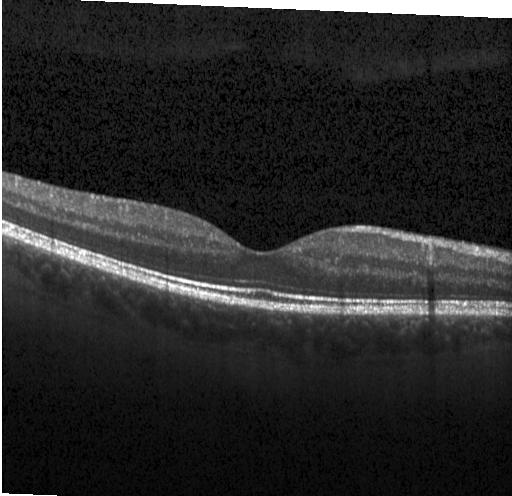
Instrument: Heidelberg Spectralis; SD-OCT; OCT B-scan; macular scan.
The scan shows no evidence of CNV, DME, or drusen.